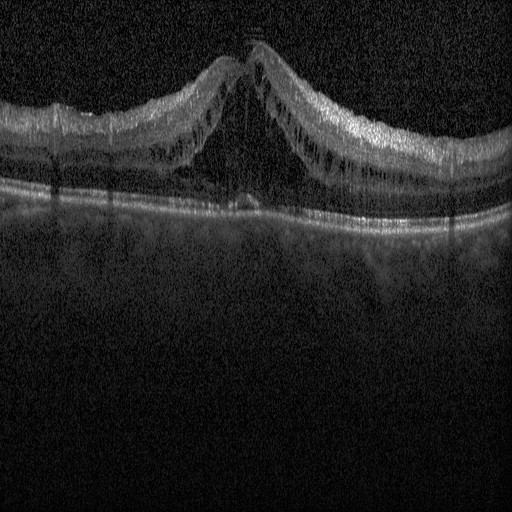
Diagnosis: DME.